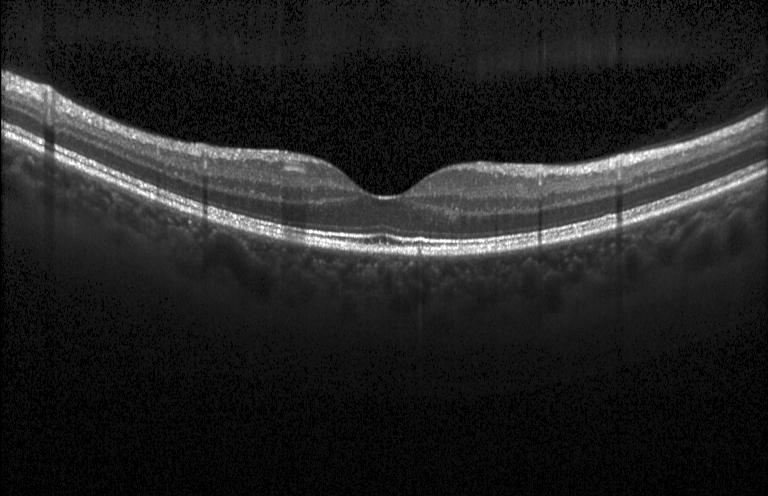 Diagnosis: neither CNV, DME, nor drusen.